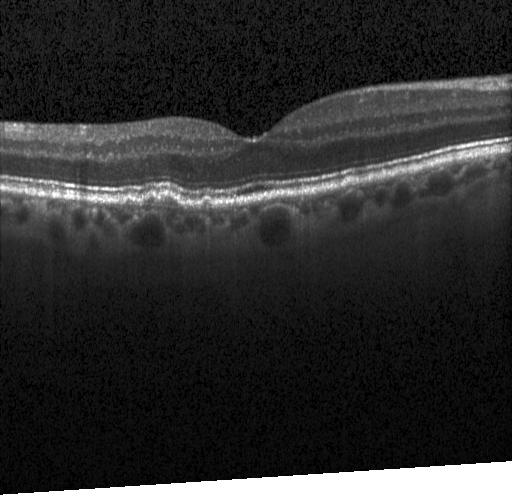
Heidelberg Spectralis; optical coherence tomography B-scan; centered on the fovea
Diagnosis: multiple drusen.